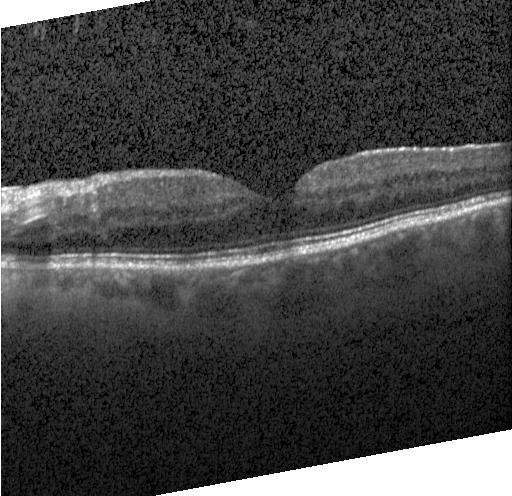 Retinal OCT B-scan. Fovea-centered
Diagnosis: no choroidal neovascularization, diabetic macular edema, or drusen.